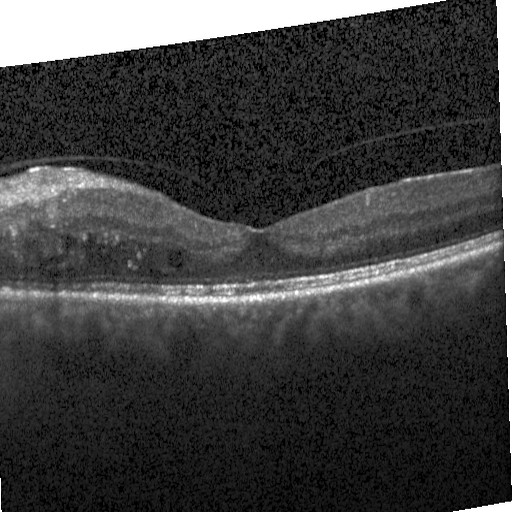

Spectral-domain OCT B-scan: DME.